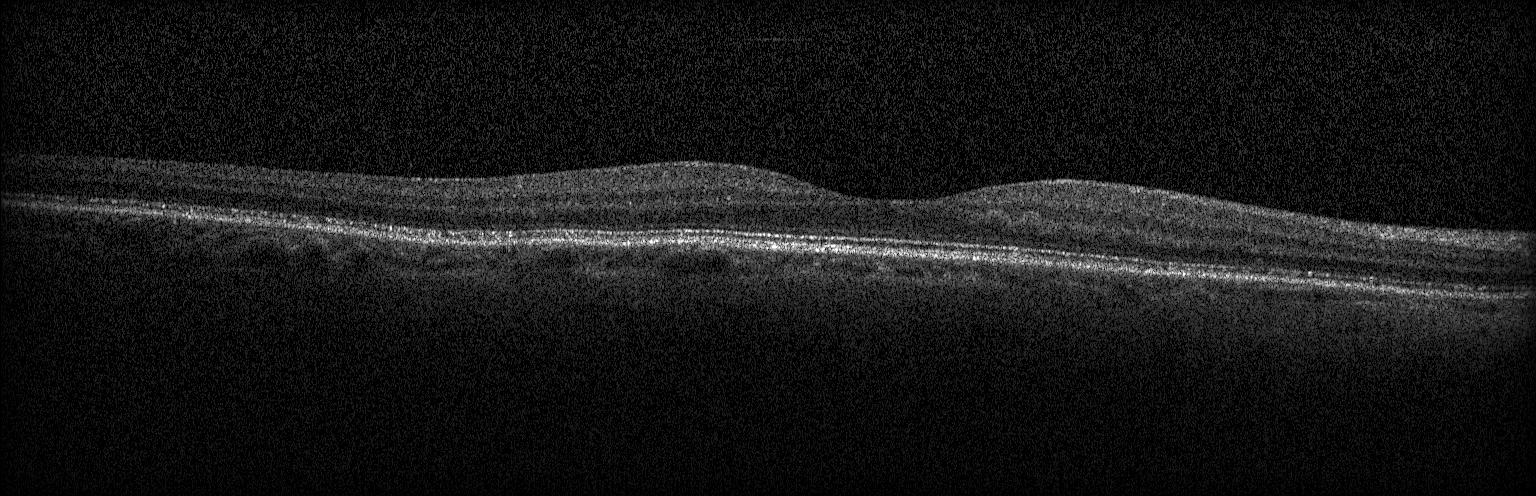

The scan shows no evidence of choroidal neovascularization, diabetic macular edema, or drusen.